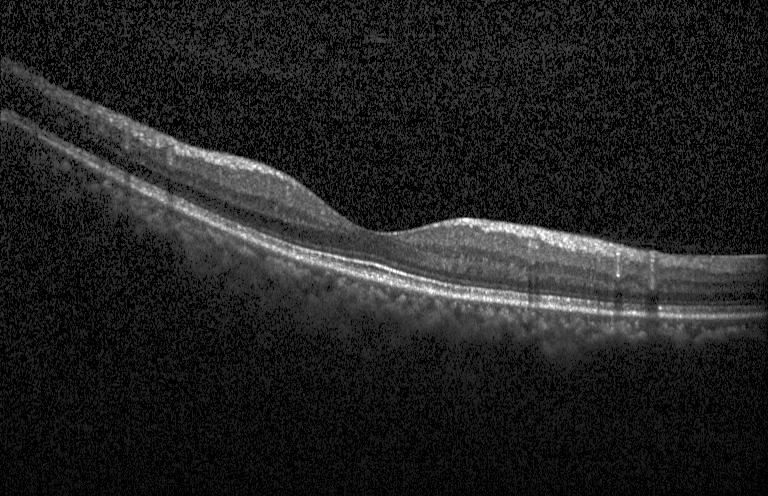
Spectral-domain OCT; through the macula; retinal OCT B-scan — Finding: no CNV, DME, or drusen.